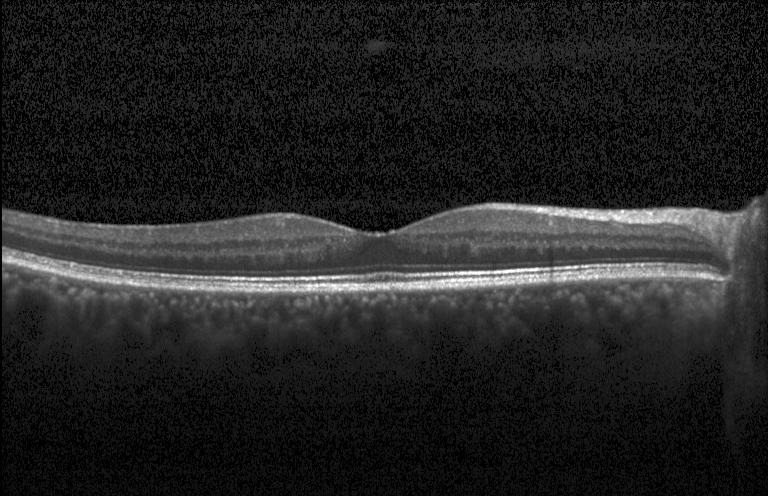

Macular OCT: no evidence of choroidal neovascularization, diabetic macular edema, or drusen.